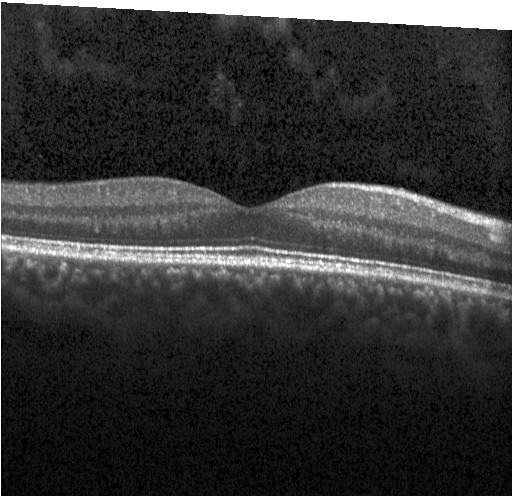
Spectral-domain OCT. Heidelberg Spectralis OCT system. Optical coherence tomography scan. Macular scan — Diagnosis: neither choroidal neovascularization, diabetic macular edema, nor drusen.